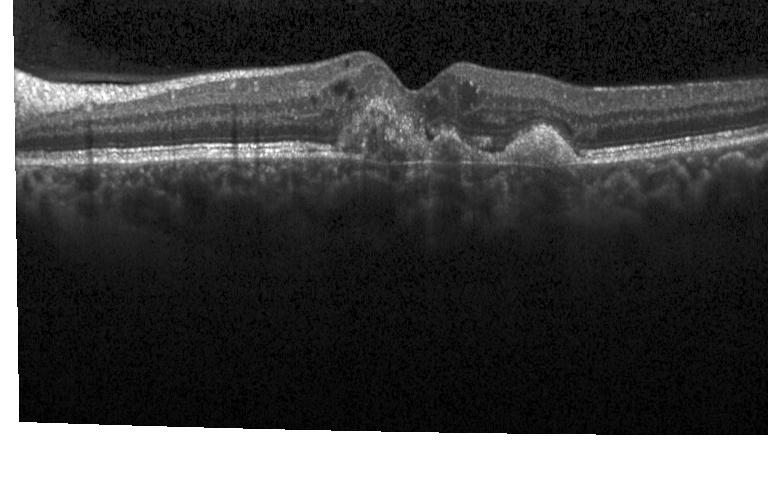 Spectral-domain OCT B-scan: a choroidal neovascular membrane.